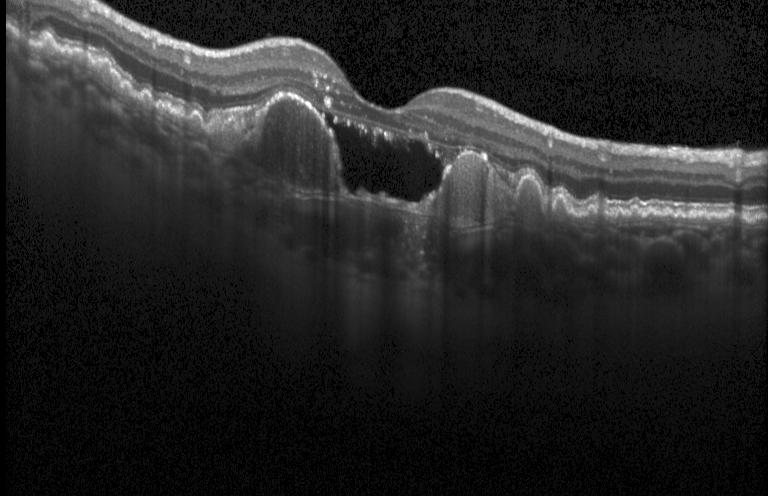

Centered on the fovea. Optical coherence tomography B-scan
This B-scan demonstrates choroidal neovascularization (CNV).